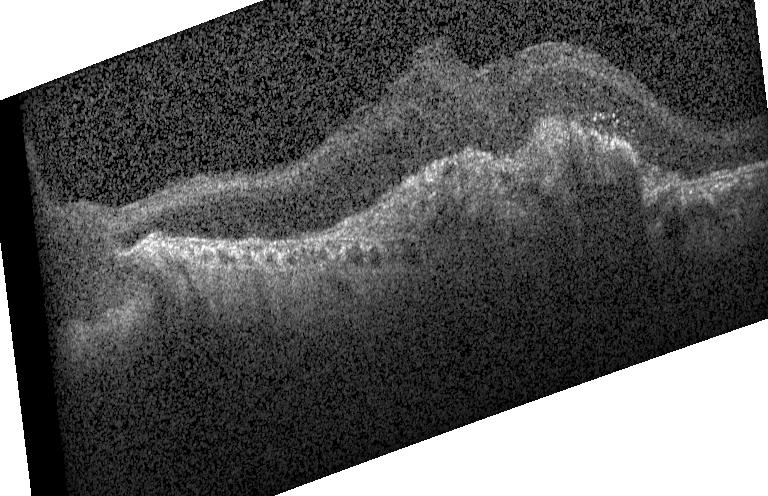 Spectral-domain optical coherence tomography. Optical coherence tomography B-scan. Heidelberg Spectralis OCT system. Fovea-centered
CNV.